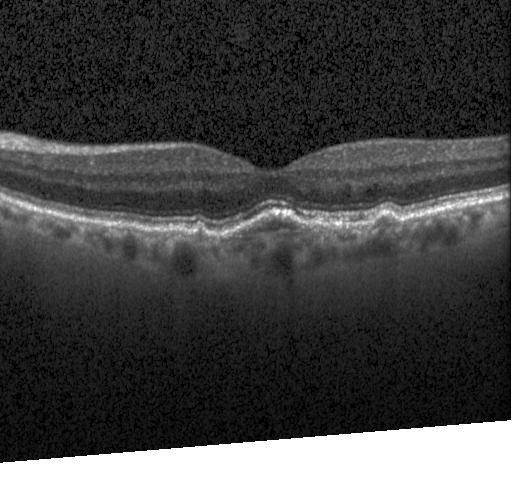

Acquired on a Heidelberg Spectralis · optical coherence tomography scan · through the macula · spectral-domain OCT
Impression: CNV.